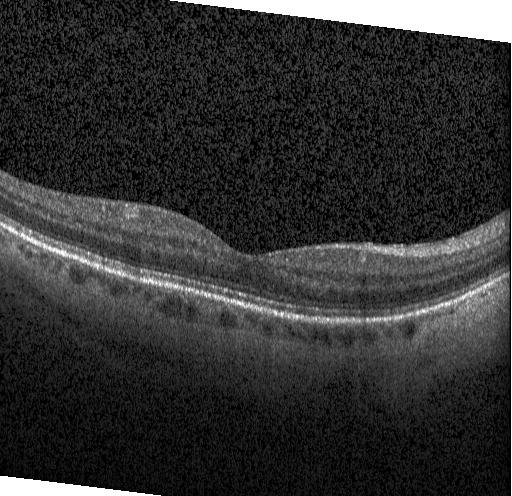
OCT line scan. Diagnosis: no choroidal neovascularization, diabetic macular edema, or drusen.